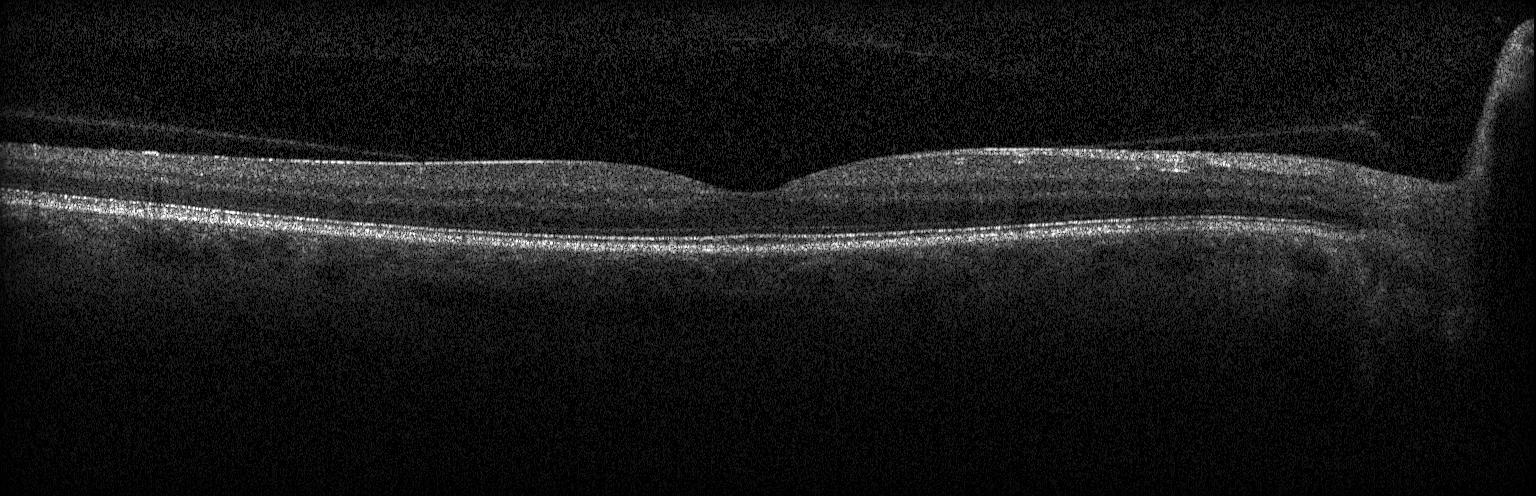
The scan shows no evidence of choroidal neovascularization, diabetic macular edema, or drusen.